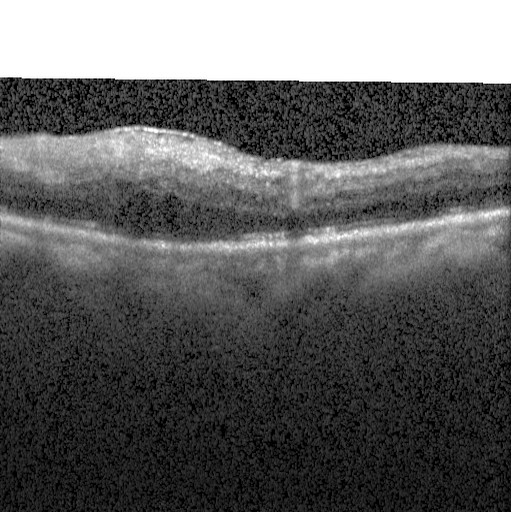
Impression: diabetic macular edema.